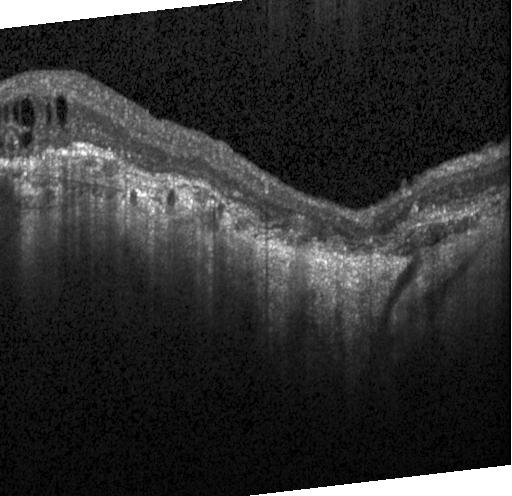 Retinal OCT cross-section showing CNV.